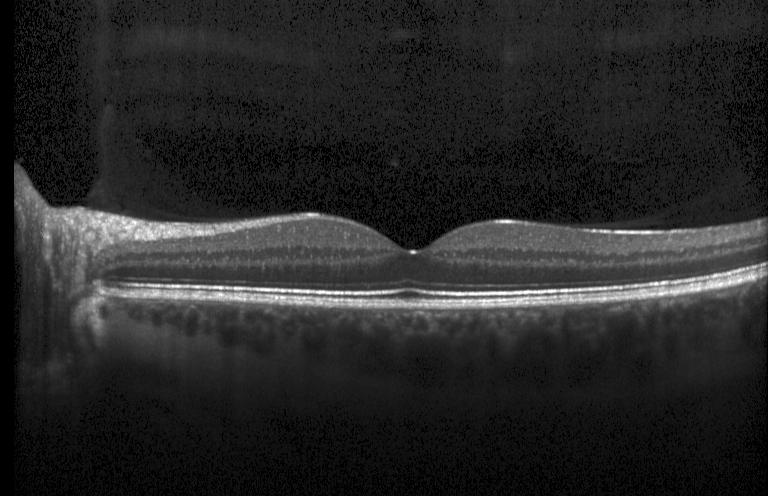
Optical coherence tomography scan — Dx: neither choroidal neovascularization, diabetic macular edema, nor drusen.